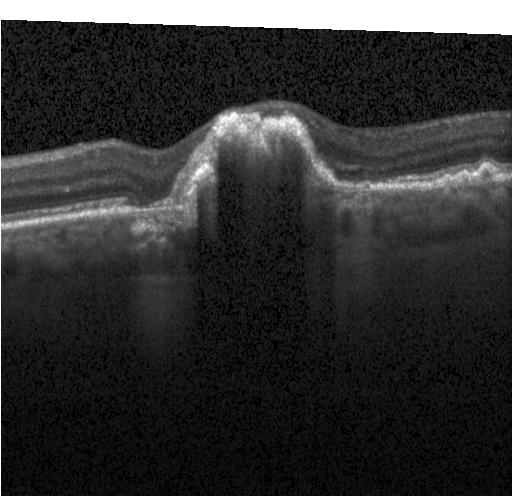
Retinal OCT cross-section; centered on the fovea; Heidelberg Spectralis; spectral-domain OCT. Dx: a choroidal neovascular membrane.